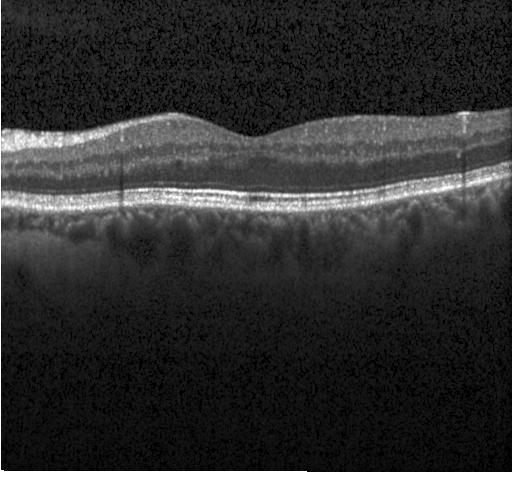 Optical coherence tomography scan · spectral-domain optical coherence tomography.
Impression: no CNV, DME, or drusen.